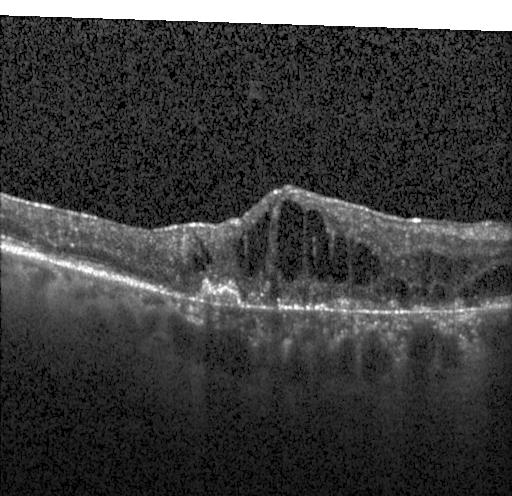 OCT scan showing choroidal neovascularization.